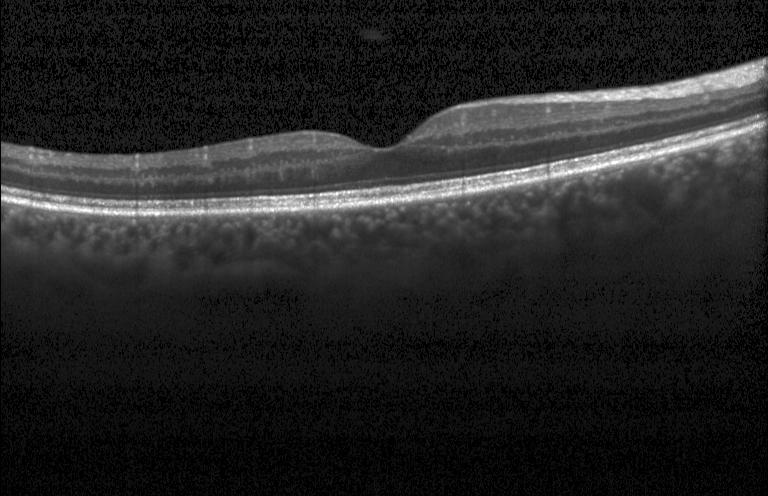
SD-OCT, optical coherence tomography scan.
Finding: neither choroidal neovascularization, diabetic macular edema, nor drusen.